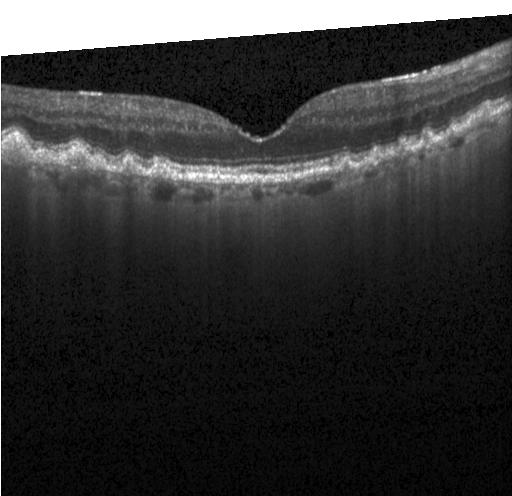

This B-scan demonstrates drusen.